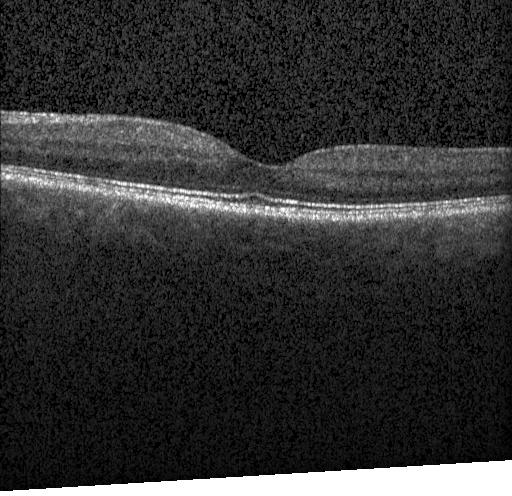 Instrument: Heidelberg Spectralis · optical coherence tomography scan · SD-OCT · macular scan. Assessment: no evidence of choroidal neovascularization, diabetic macular edema, or drusen.